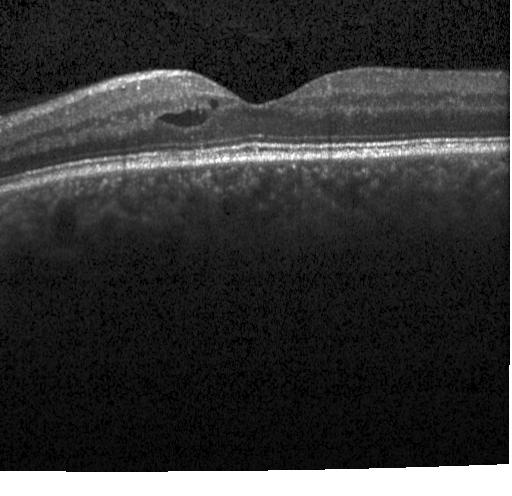 Impression: DME.